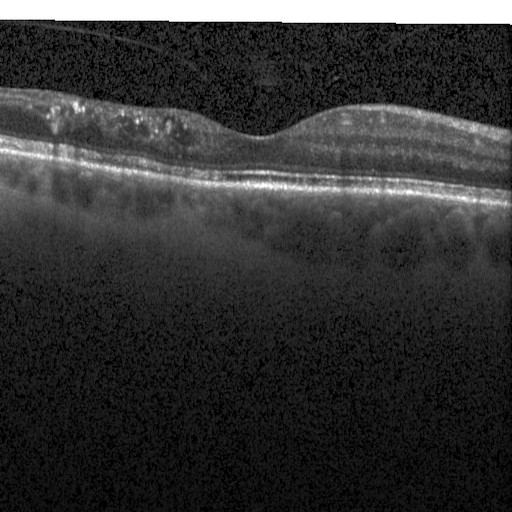

Spectral-domain optical coherence tomography; through the macula; retinal OCT cross-section.
Impression: diabetic macular edema (DME).